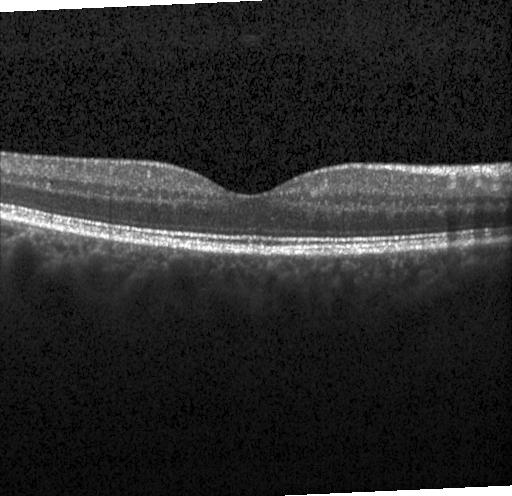

OCT line scan
Diagnosis: neither choroidal neovascularization, diabetic macular edema, nor drusen.